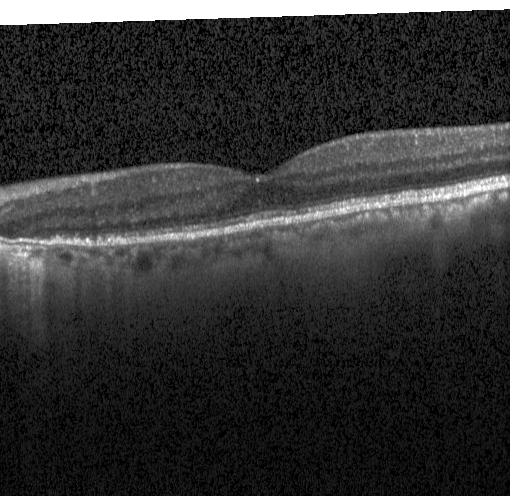
Optical coherence tomography B-scan. Assessment: no CNV, no DME, and no drusen.